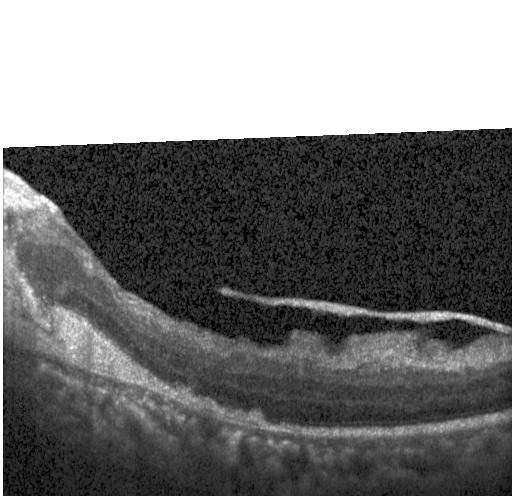

Through the macula, OCT B-scan — Dx: a choroidal neovascular membrane.